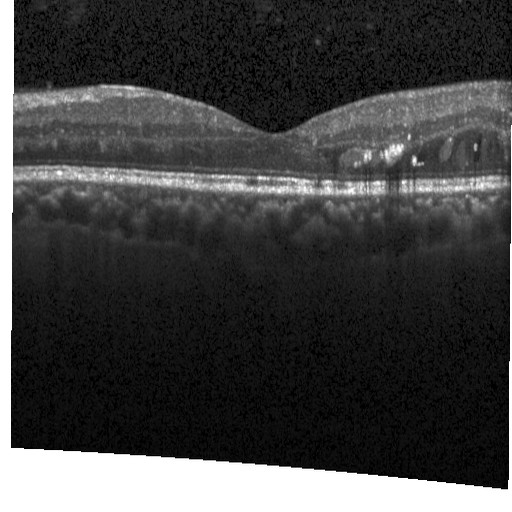

Macular scan. Optical coherence tomography B-scan. SD-OCT.
Finding: diabetic macular edema (DME).